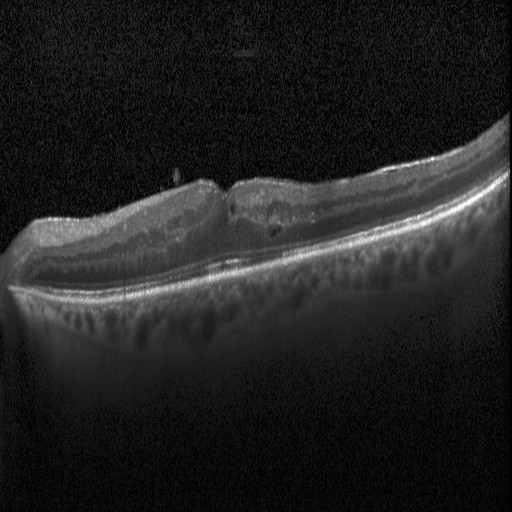

Heidelberg Spectralis · spectral-domain OCT · centered on the fovea · OCT B-scan
Diagnosis: diabetic macular edema.